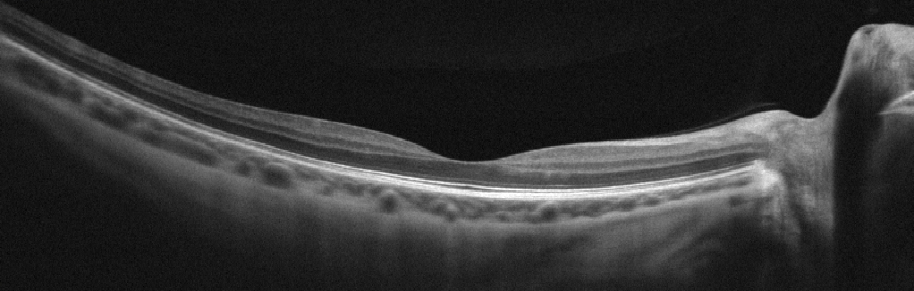 Macular scan, optical coherence tomography B-scan, Optovue Avanti RTVue XR
Diagnosis: absence of AMD, DME, ERM, RAO, RVO, and vitreomacular interface disease.